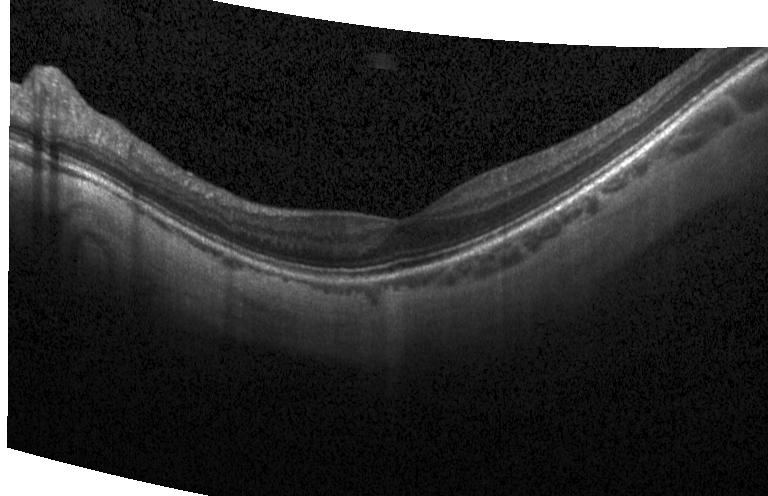 Optical coherence tomography scan · horizontal scan through the fovea — Finding: no evidence of choroidal neovascularization, diabetic macular edema, or drusen.